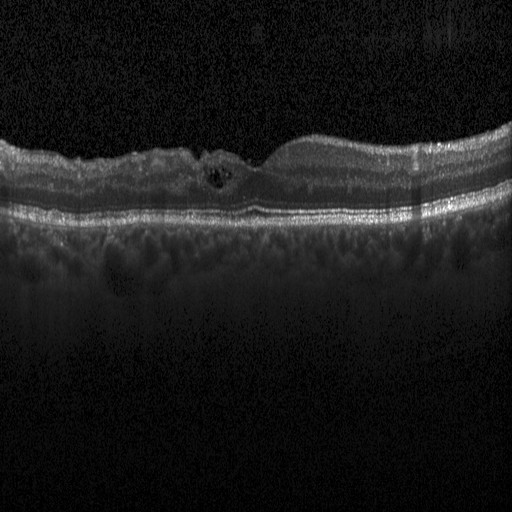

Instrument: Heidelberg Spectralis. Optical coherence tomography B-scan. Impression: DME.